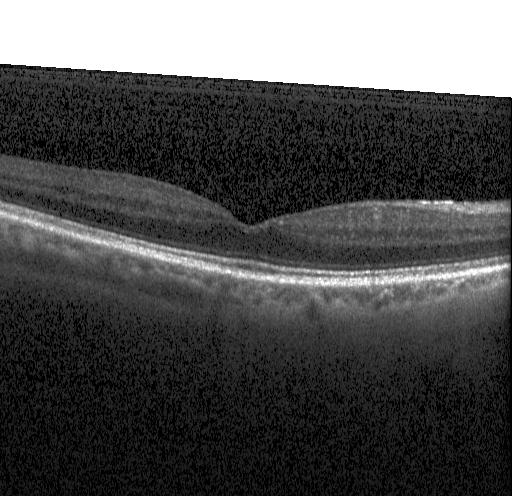

OCT finding: neither CNV, DME, nor drusen.